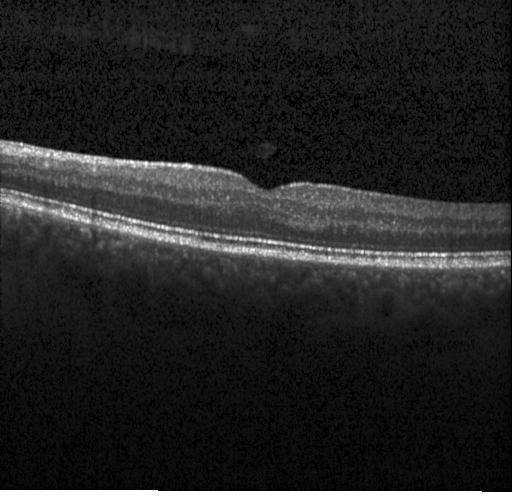 Assessment: no choroidal neovascularization, no diabetic macular edema, and no drusen.